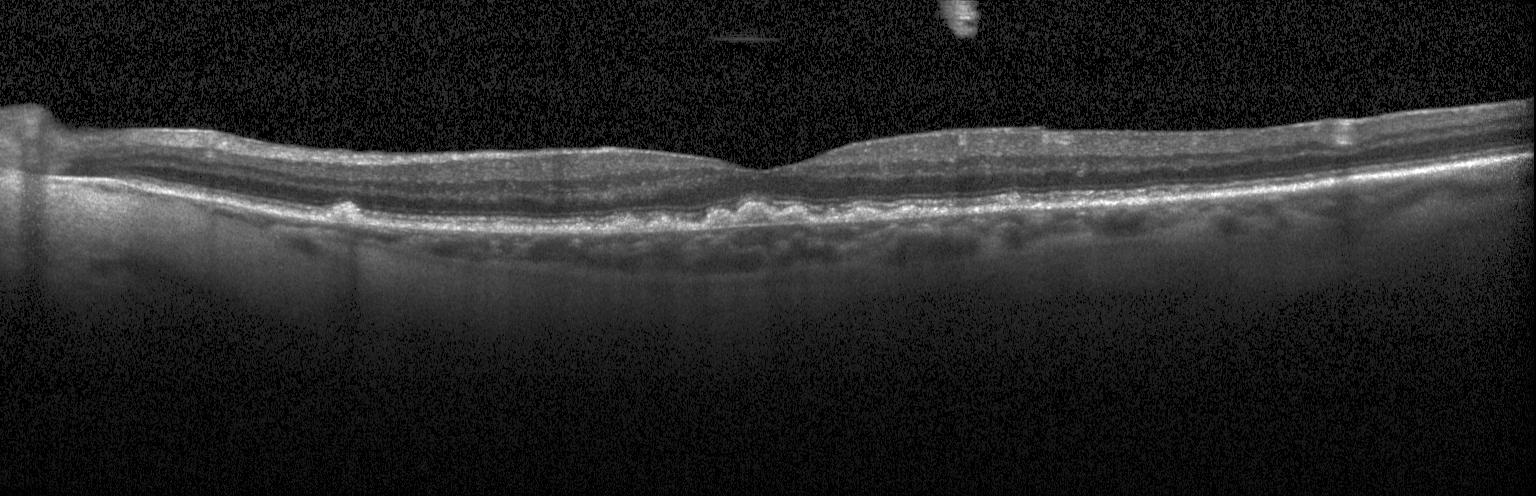
Optical coherence tomography scan; SD-OCT
OCT finding: sub-RPE drusenoid deposits.